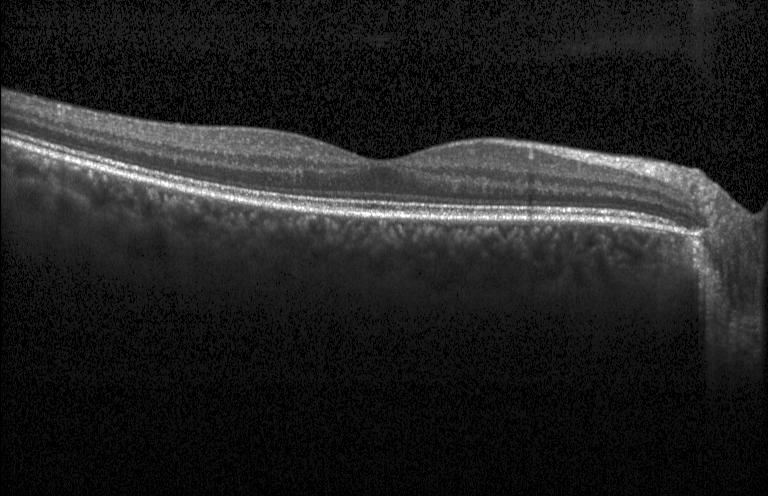 Spectral-domain OCT B-scan: no choroidal neovascularization, no diabetic macular edema, and no drusen.